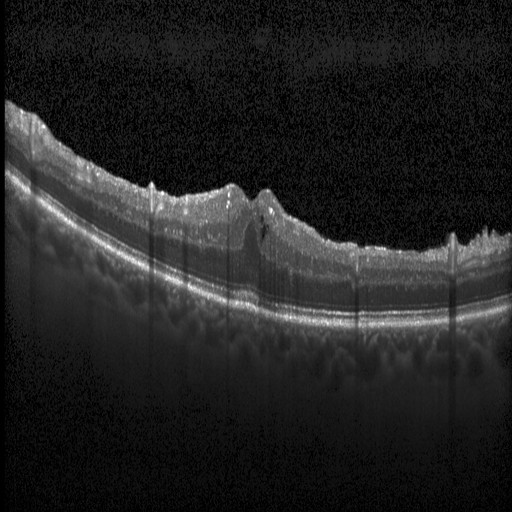 SD-OCT; macular scan; optical coherence tomography scan; Heidelberg Spectralis — Macular OCT: diabetic macular edema.